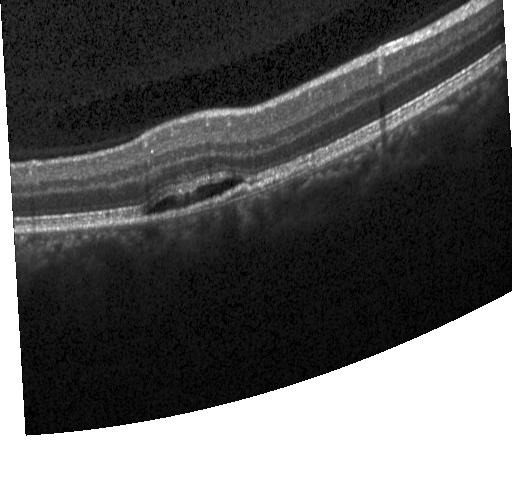
Optical coherence tomography B-scan · Heidelberg Spectralis · through the macula.
Diagnosis: a choroidal neovascular membrane.